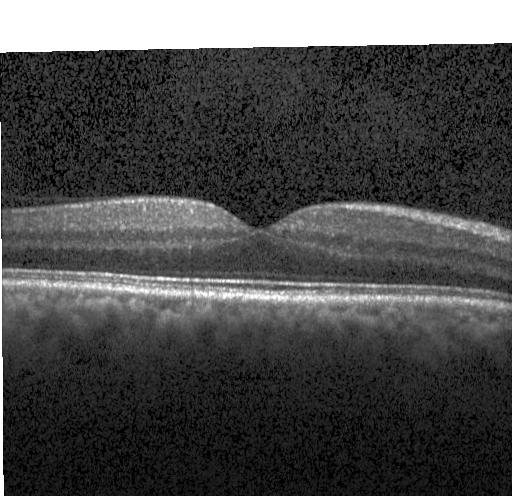
OCT line scan. Diagnosis: no evidence of CNV, DME, or drusen.